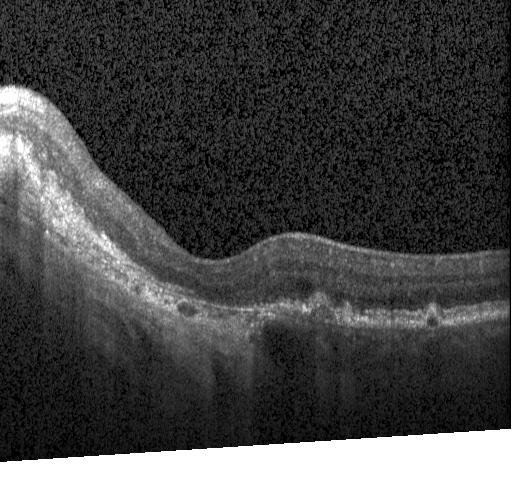
Assessment: CNV.